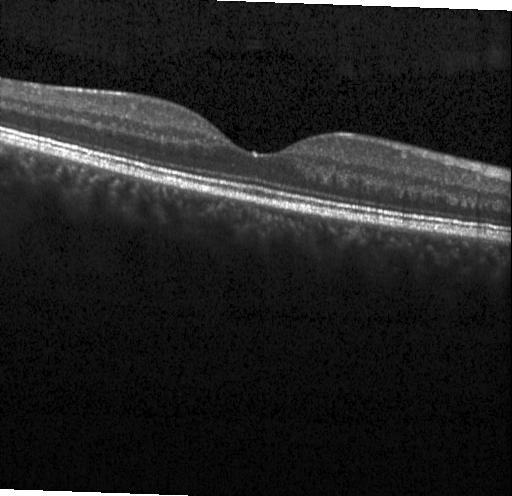 SD-OCT · OCT line scan. Assessment: neither choroidal neovascularization, diabetic macular edema, nor drusen.